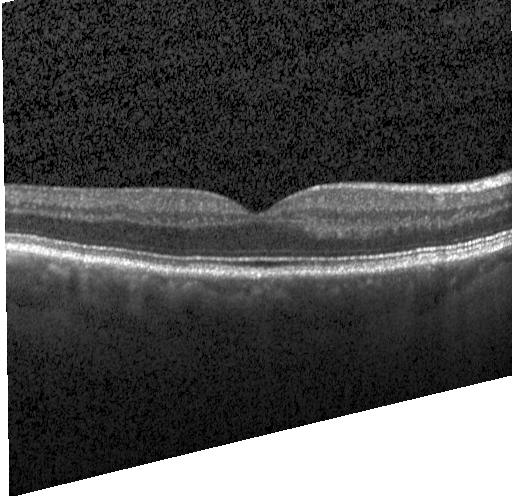

Optical coherence tomography B-scan. SD-OCT. Through the macula. Assessment: neither choroidal neovascularization, diabetic macular edema, nor drusen.